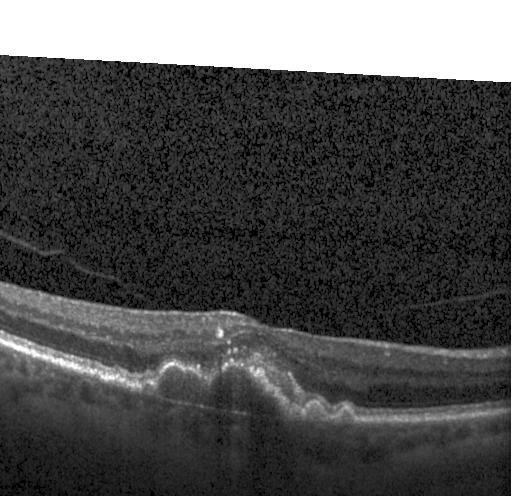
The scan shows a choroidal neovascular membrane.